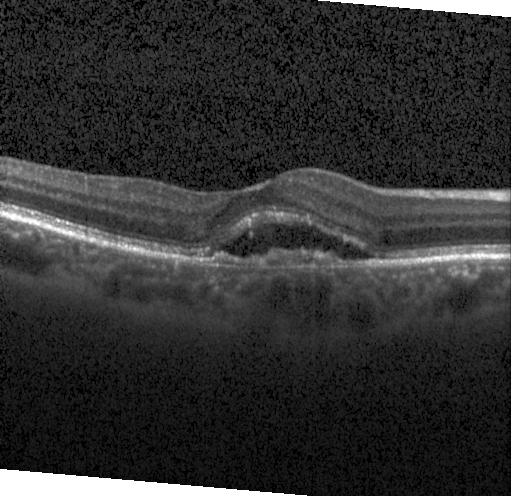

Impression: CNV.